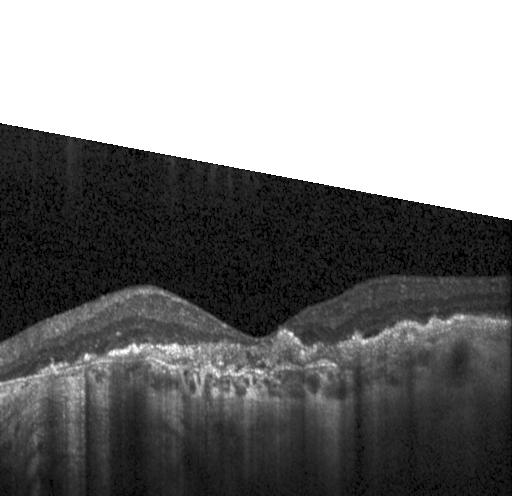 Retinal OCT B-scan; spectral-domain OCT; macular scan.
Diagnosis: choroidal neovascularization (CNV).